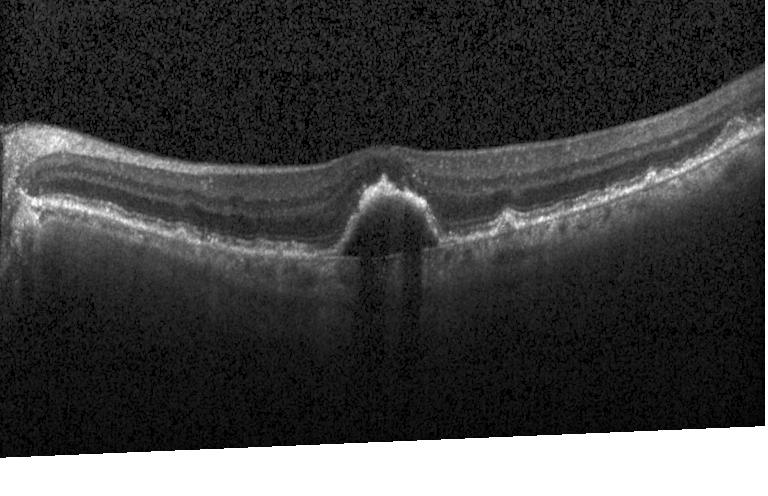 OCT scan showing a choroidal neovascular membrane.